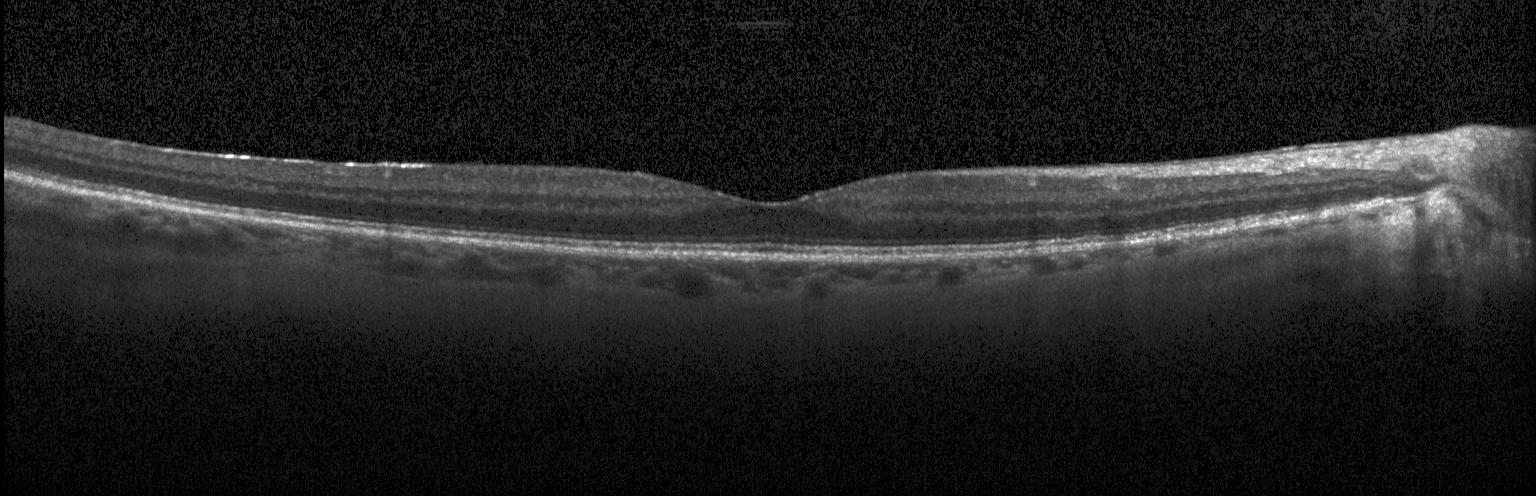
Centered on the fovea. Spectral-domain OCT. OCT line scan.
Finding: neither choroidal neovascularization, diabetic macular edema, nor drusen.